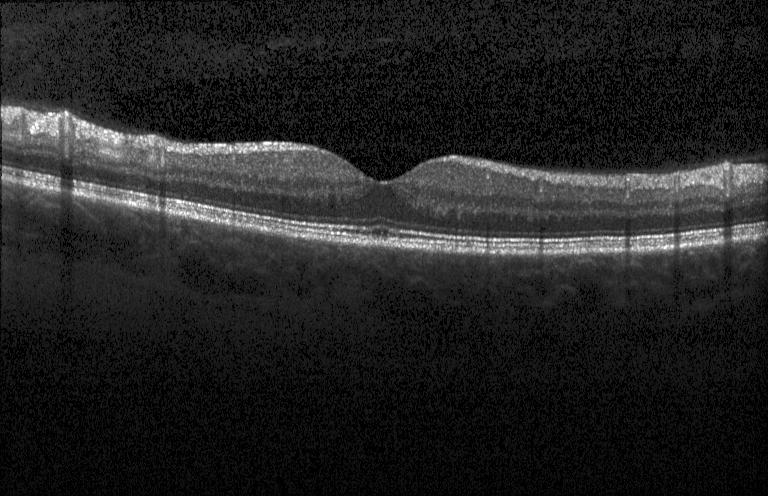
OCT line scan
Impression: no CNV, DME, or drusen.